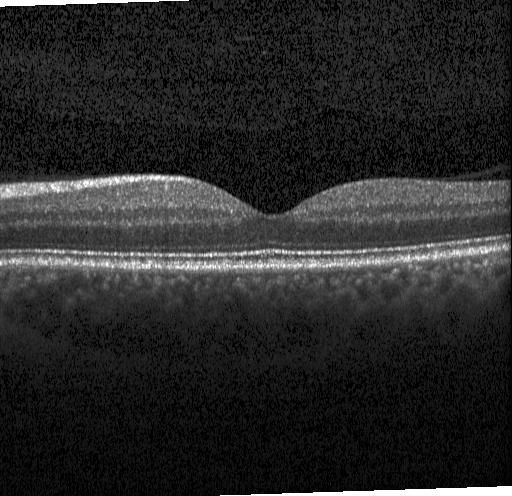
Fovea-centered. Heidelberg Spectralis. Retinal OCT B-scan — Diagnosis: no CNV, no DME, and no drusen.